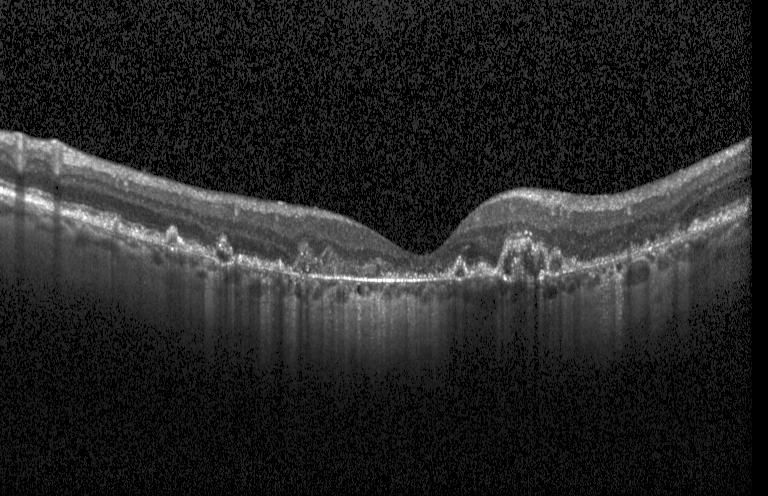

OCT B-scan showing a choroidal neovascular membrane.